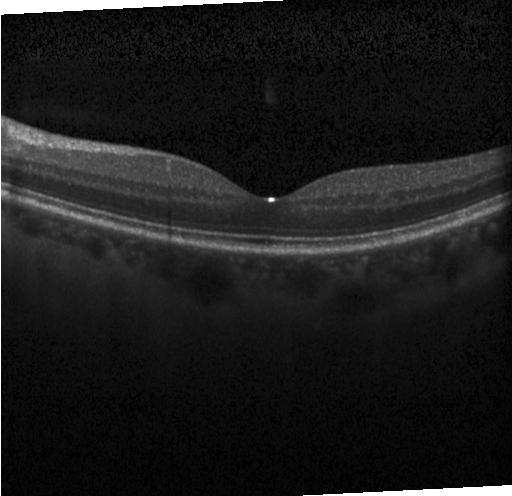 Finding: no choroidal neovascularization, no diabetic macular edema, and no drusen.